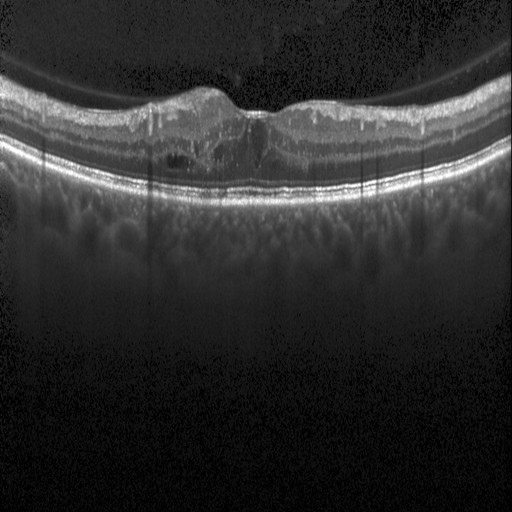
Impression: diabetic macular edema.